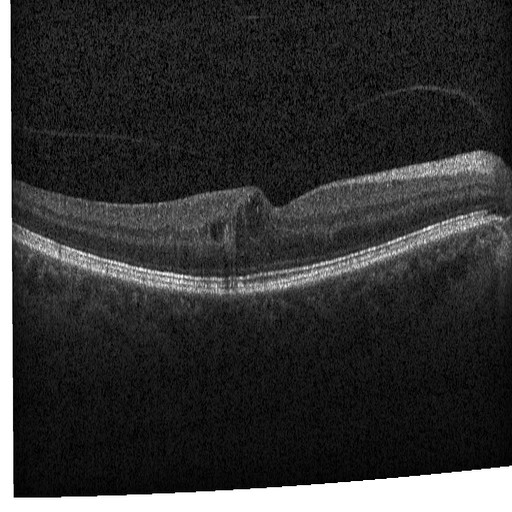 Centered on the fovea; optical coherence tomography scan.
This B-scan demonstrates diabetic macular edema.